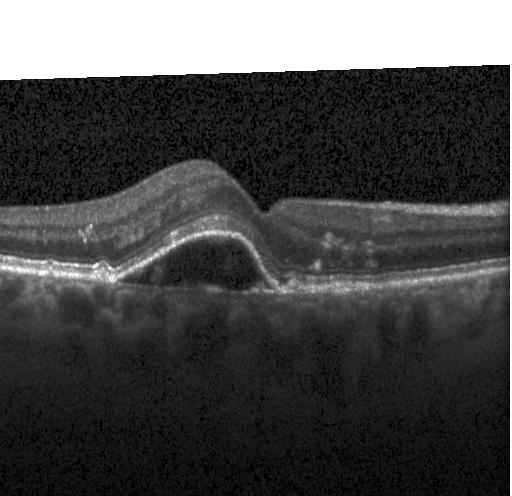

SD-OCT · retinal OCT B-scan
This B-scan demonstrates a choroidal neovascular membrane.